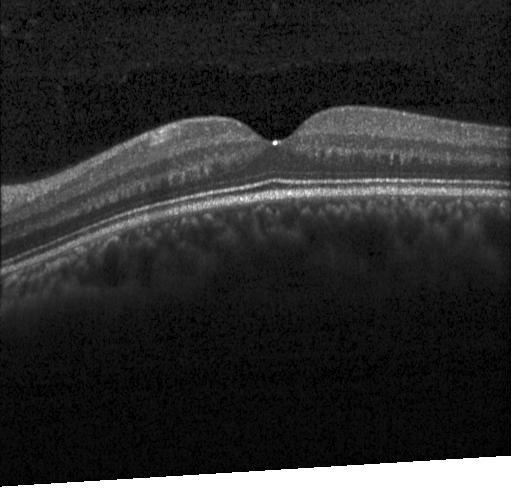

Impression: neither choroidal neovascularization, diabetic macular edema, nor drusen.